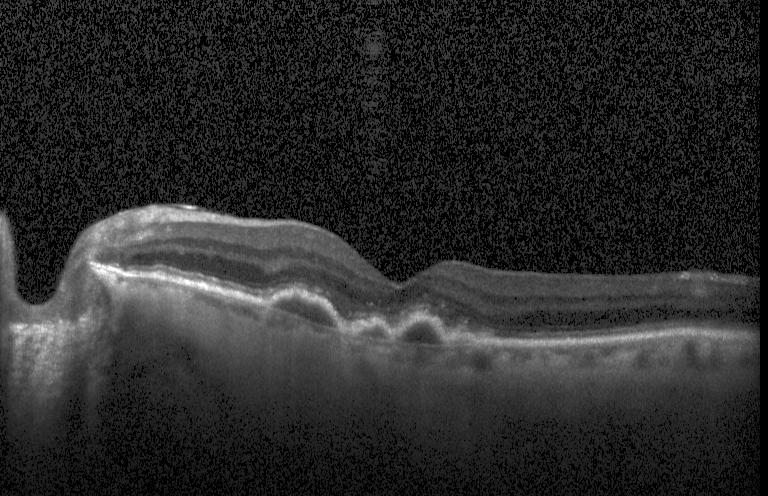 Macular OCT demonstrating CNV.